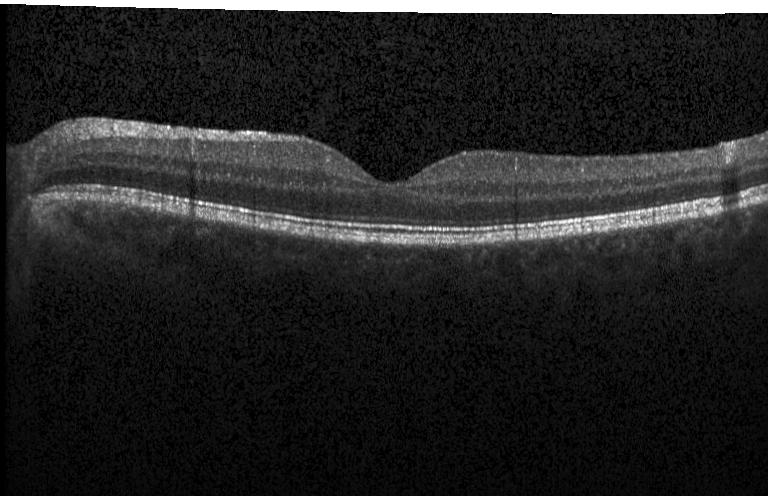 Dx: no evidence of choroidal neovascularization, diabetic macular edema, or drusen.